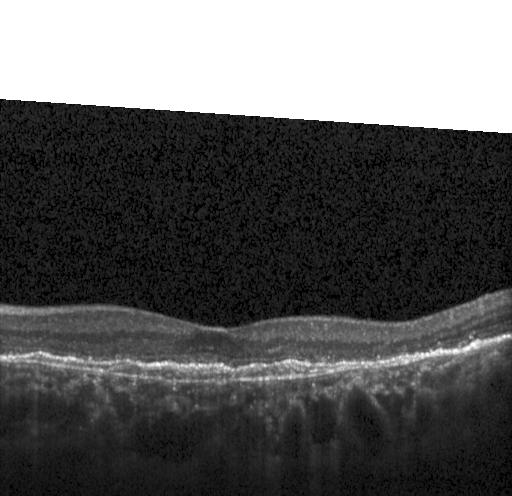 Impression: a choroidal neovascular membrane.